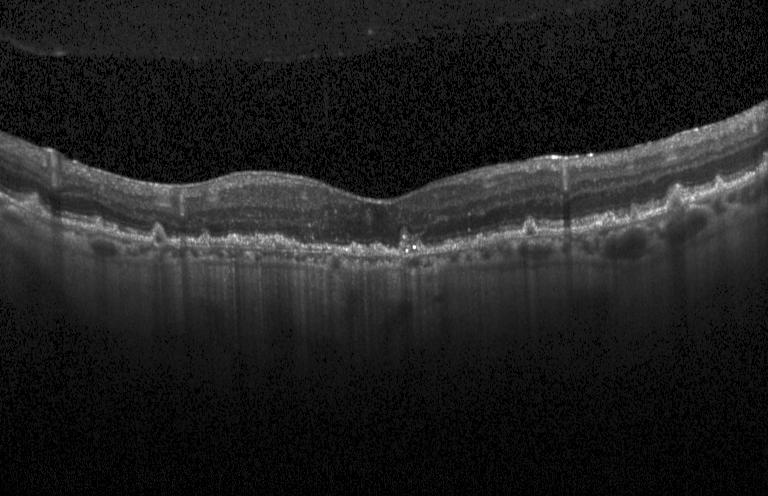

Acquired on a Heidelberg Spectralis. OCT B-scan. Spectral-domain optical coherence tomography
Diagnosis: a choroidal neovascular membrane.